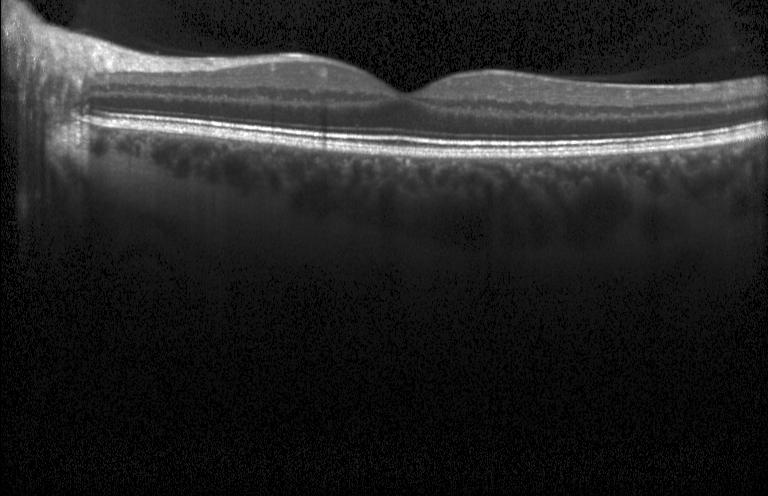

Macular OCT: no choroidal neovascularization, diabetic macular edema, or drusen.